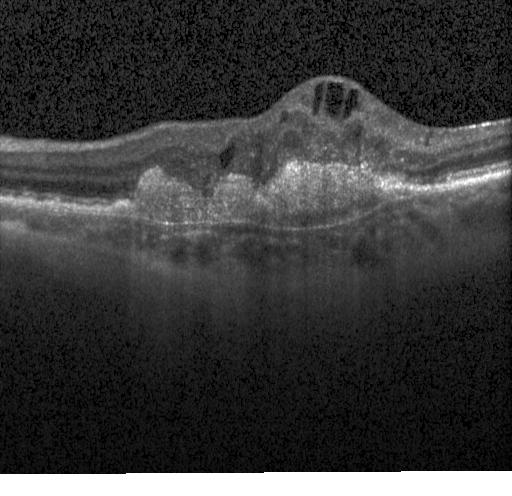
Impression: choroidal neovascularization (CNV).